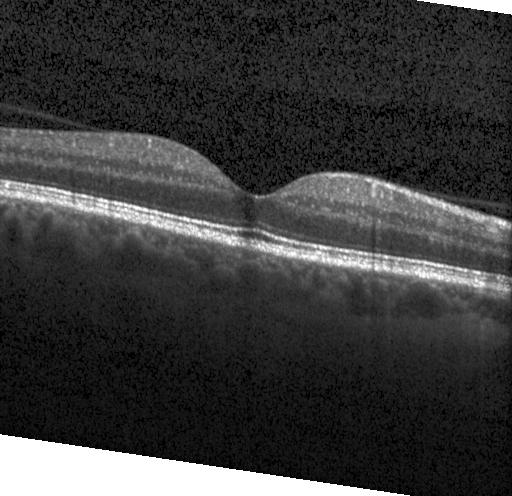 Spectral-domain OCT; OCT line scan
Diagnosis: no evidence of choroidal neovascularization, diabetic macular edema, or drusen.